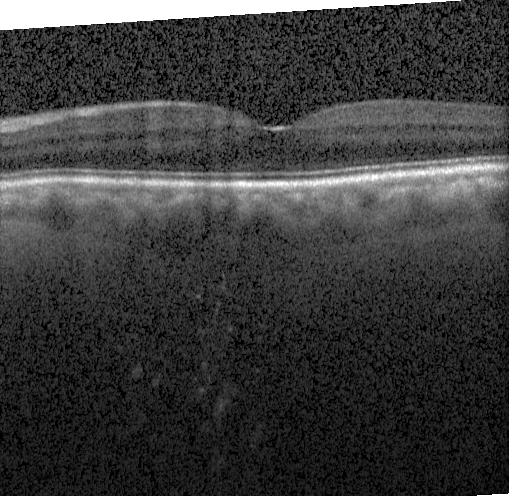 Acquired on a Heidelberg Spectralis; centered on the fovea; OCT line scan
Diagnosis: no evidence of CNV, DME, or drusen.